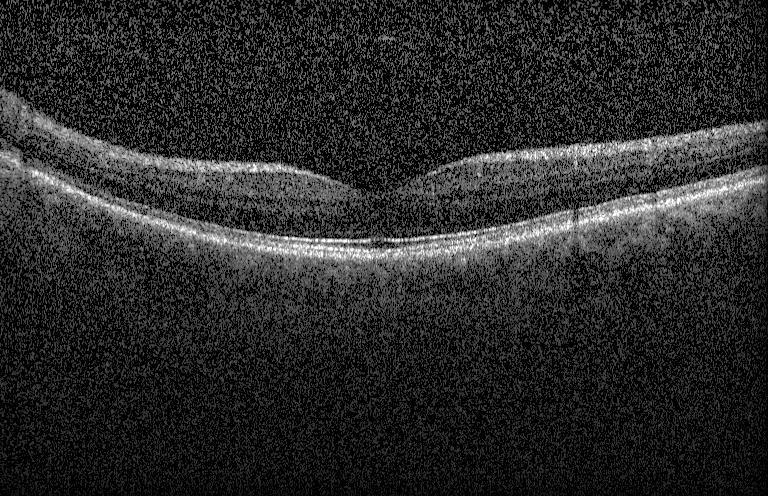
The scan shows neither CNV, DME, nor drusen.